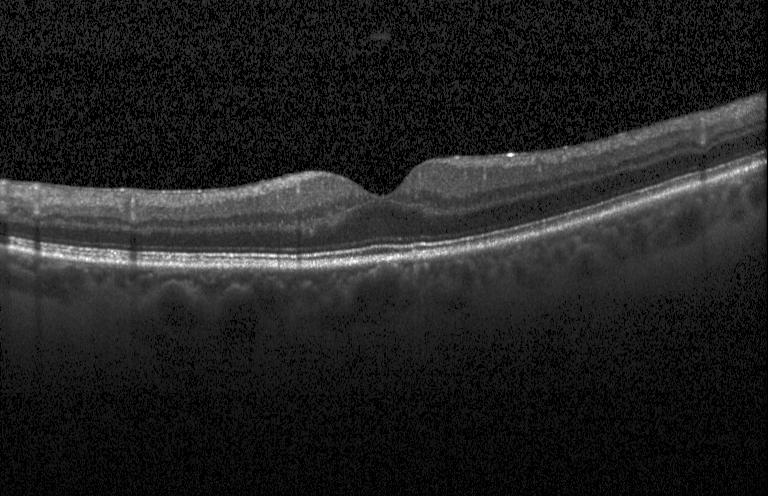 Spectral-domain optical coherence tomography · Heidelberg Spectralis OCT system · optical coherence tomography B-scan · fovea-centered — This B-scan demonstrates no choroidal neovascularization, no diabetic macular edema, and no drusen.